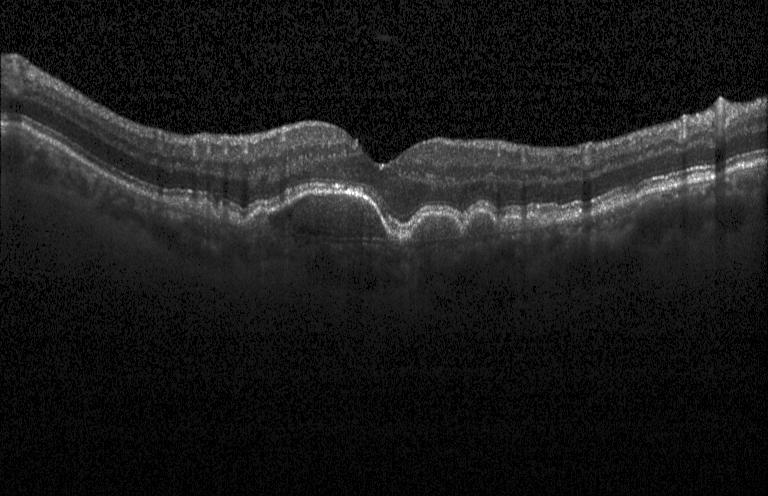
Impression: sub-RPE drusenoid deposits.